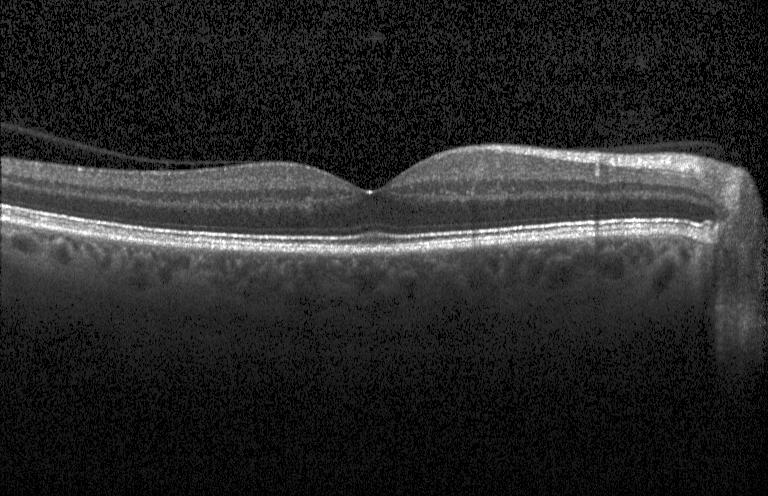
OCT line scan — Finding: no choroidal neovascularization, no diabetic macular edema, and no drusen.